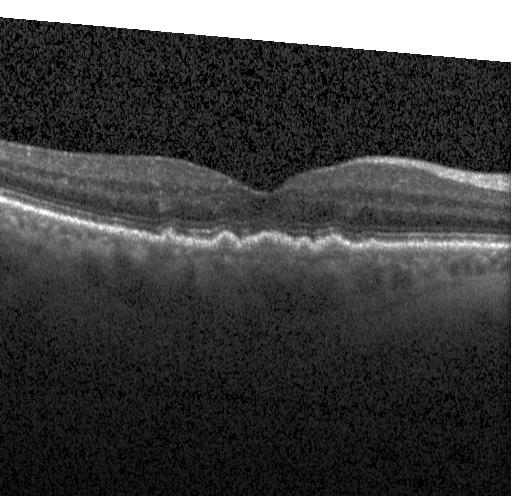
Retinal OCT cross-section; SD-OCT.
Dx: multiple drusen.